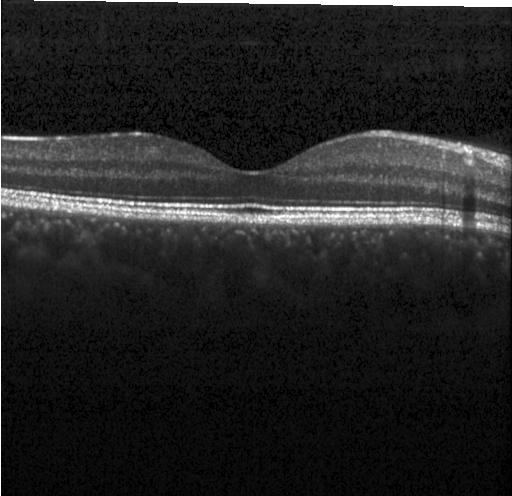
Horizontal scan through the fovea · retinal OCT cross-section · acquired on a Heidelberg Spectralis · SD-OCT — This B-scan demonstrates no CNV, no DME, and no drusen.